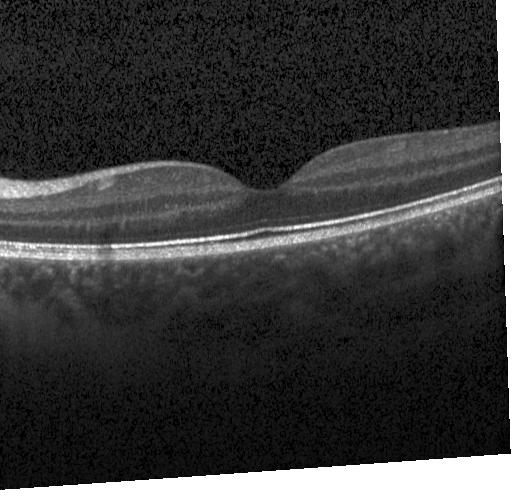

Spectral-domain OCT B-scan: neither choroidal neovascularization, diabetic macular edema, nor drusen.